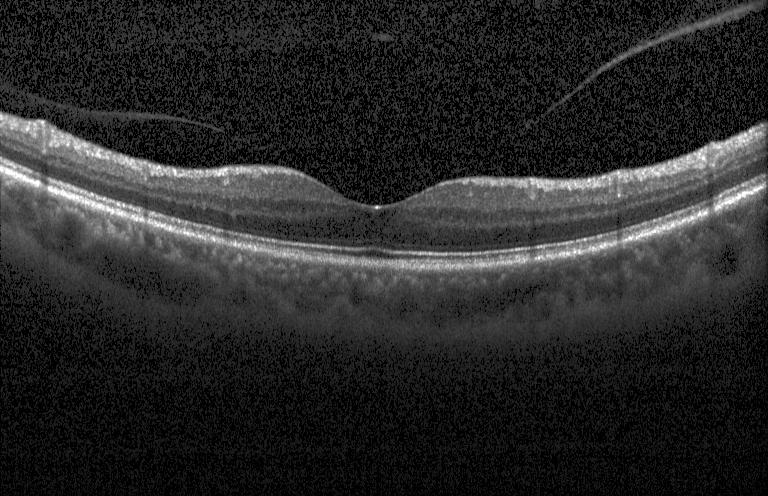
Fovea-centered. SD-OCT. Instrument: Heidelberg Spectralis. Optical coherence tomography scan — Diagnosis: neither choroidal neovascularization, diabetic macular edema, nor drusen.